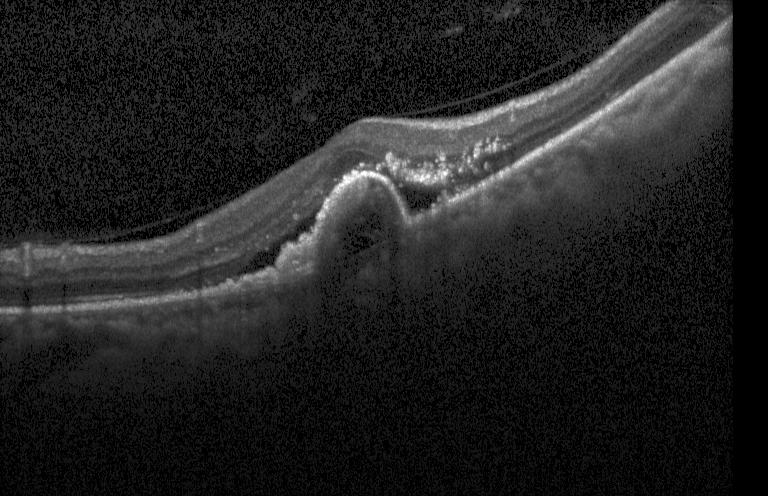
SD-OCT; fovea-centered; OCT line scan; instrument: Heidelberg Spectralis — Finding: choroidal neovascularization (CNV).